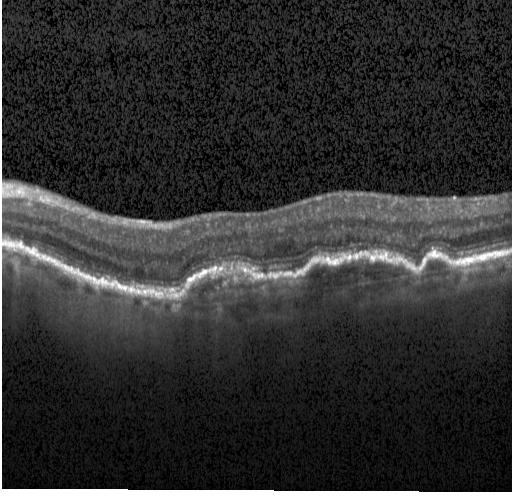 Finding: CNV.